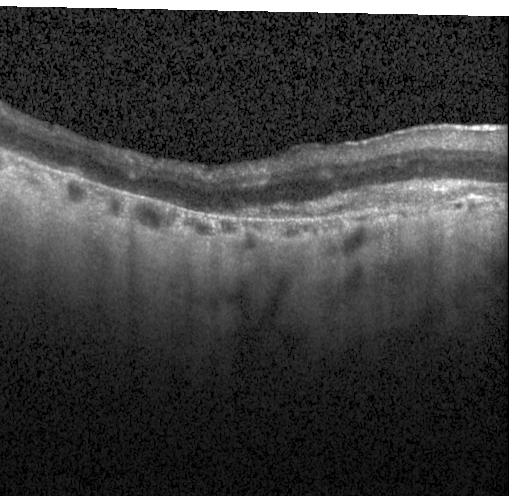

Impression: choroidal neovascularization.